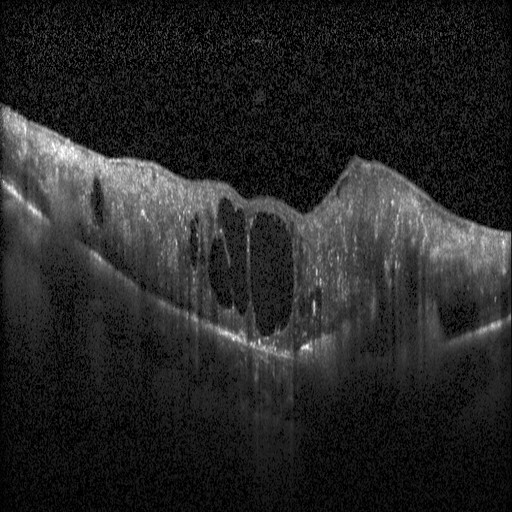
Spectral-domain OCT B-scan: diabetic macular edema (DME).